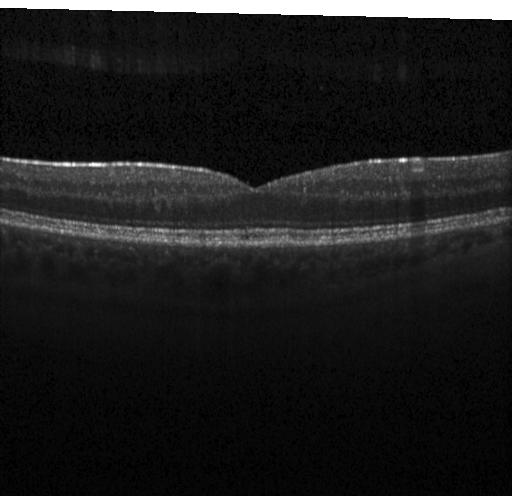
Diagnosis: no CNV, no DME, and no drusen.